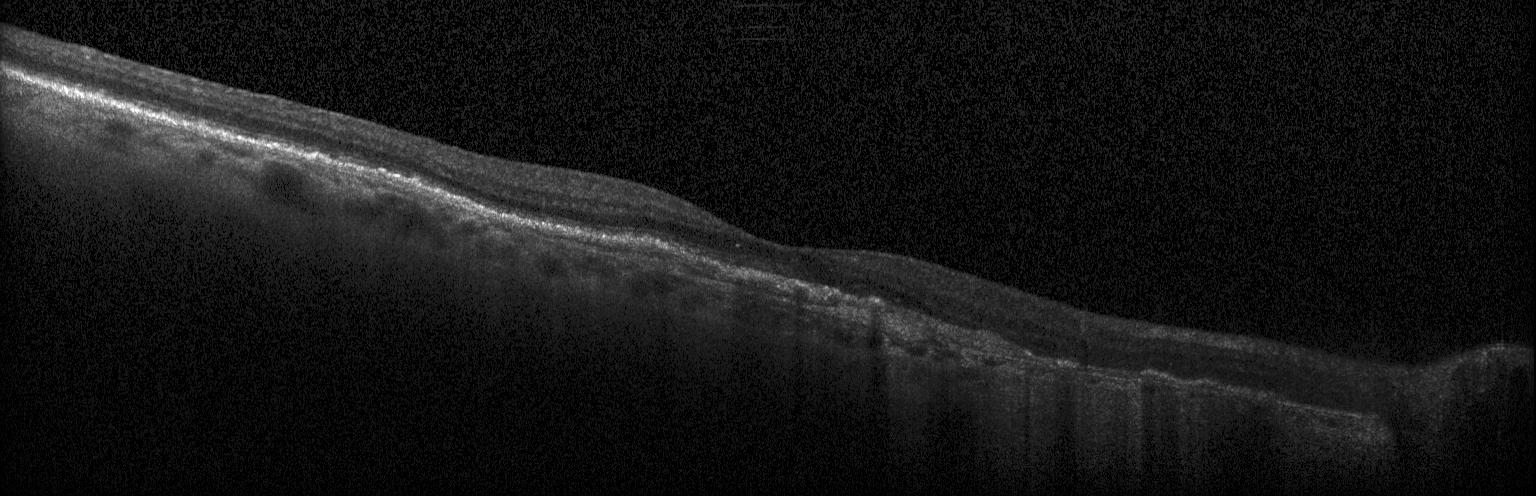

Instrument: Heidelberg Spectralis · horizontal scan through the fovea · optical coherence tomography B-scan
Assessment: choroidal neovascularization (CNV).